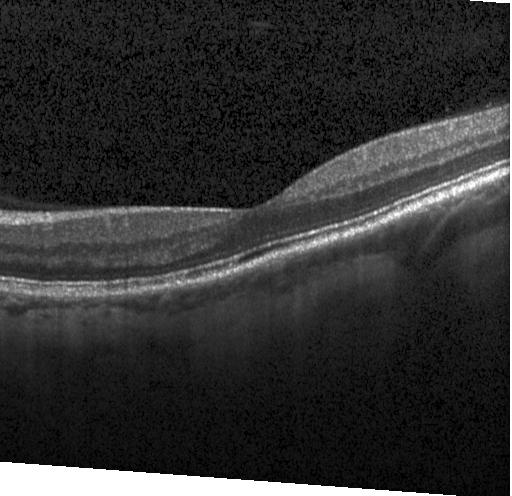 Fovea-centered, OCT line scan, spectral-domain optical coherence tomography, acquired on a Heidelberg Spectralis — Dx: no choroidal neovascularization, diabetic macular edema, or drusen.